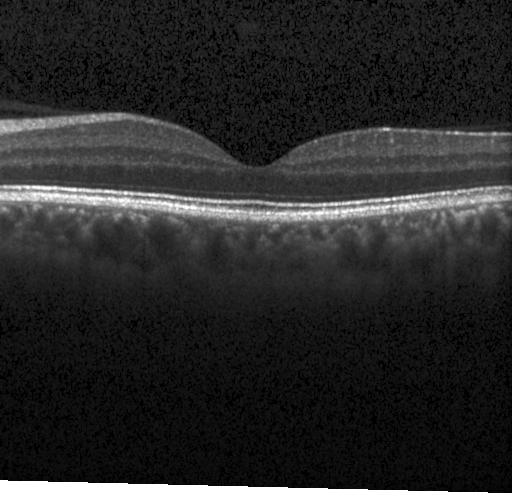
Impression: no CNV, no DME, and no drusen.